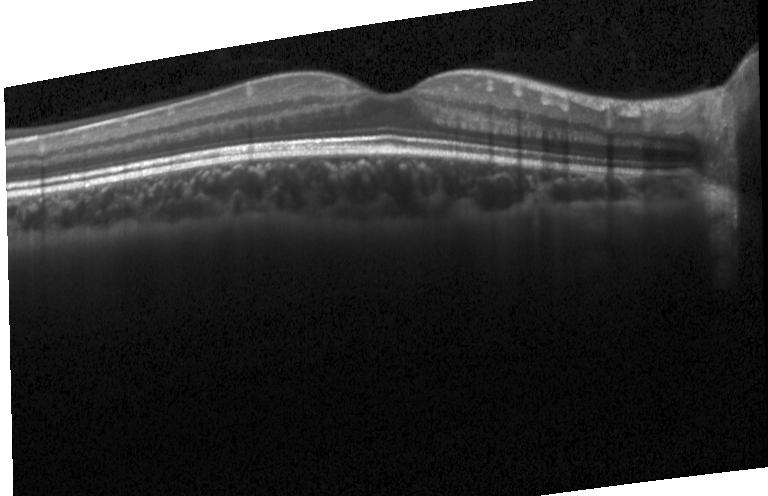
This B-scan demonstrates neither choroidal neovascularization, diabetic macular edema, nor drusen.